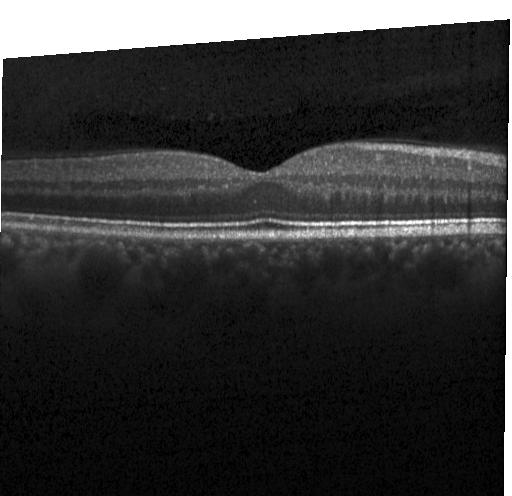
No choroidal neovascularization, diabetic macular edema, or drusen.